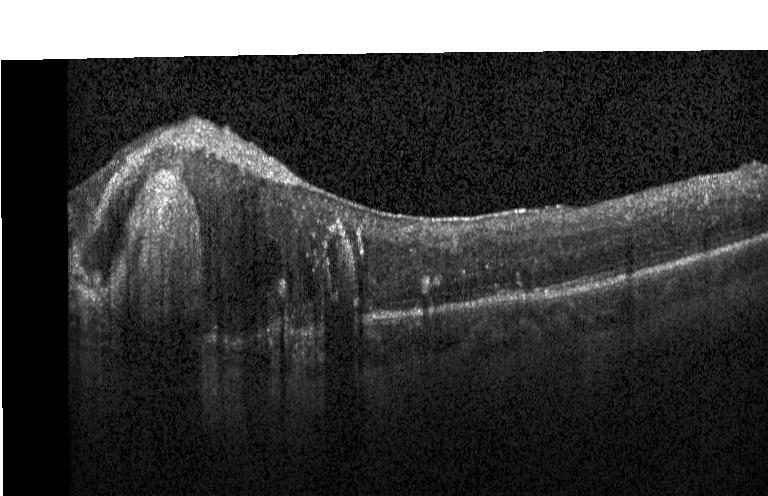
OCT finding: a choroidal neovascular membrane.